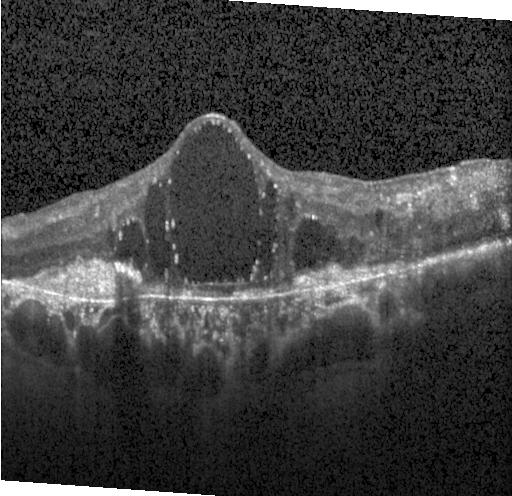

OCT line scan, macular scan, SD-OCT — Assessment: choroidal neovascularization.